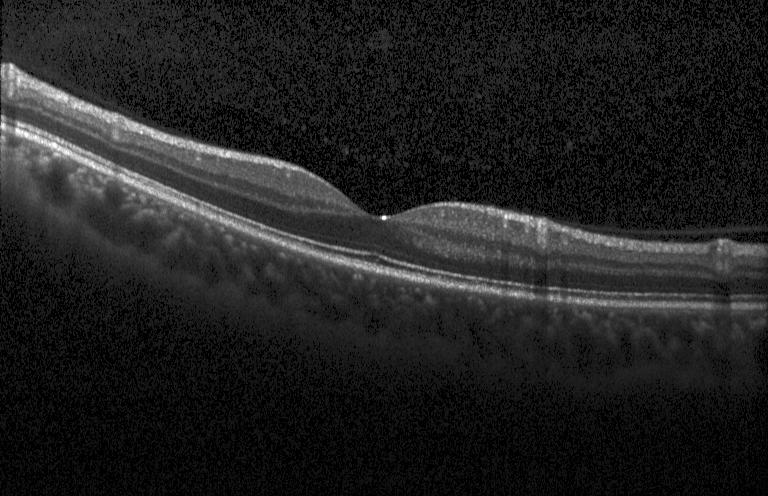
Through the macula. SD-OCT. Retinal OCT cross-section. Heidelberg Spectralis OCT system. The scan shows neither choroidal neovascularization, diabetic macular edema, nor drusen.